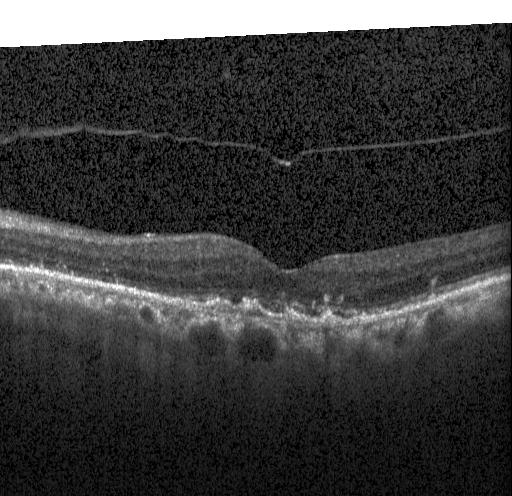
Optical coherence tomography B-scan, SD-OCT — Finding: CNV.